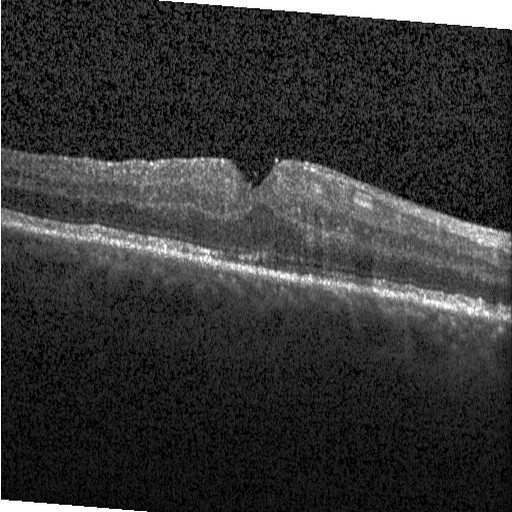
Finding: DME.